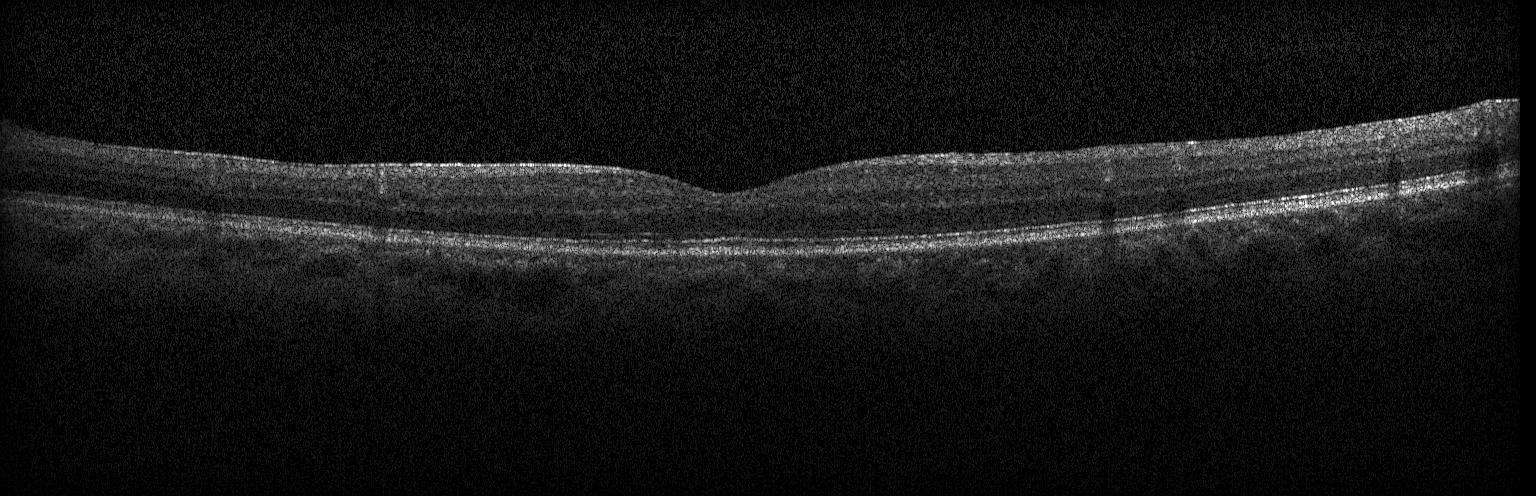
Assessment: no evidence of choroidal neovascularization, diabetic macular edema, or drusen.